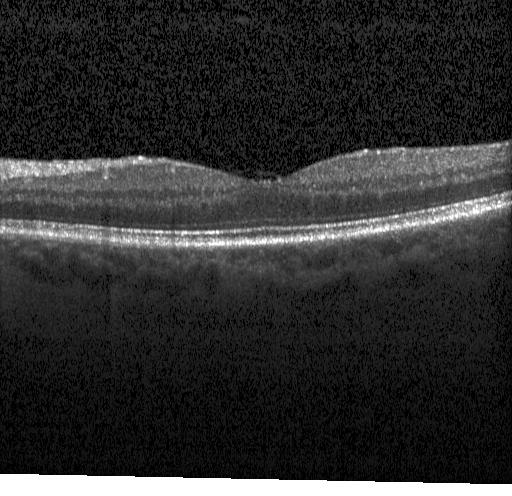 Retinal OCT cross-section, Heidelberg Spectralis, spectral-domain optical coherence tomography, fovea-centered
OCT finding: neither choroidal neovascularization, diabetic macular edema, nor drusen.